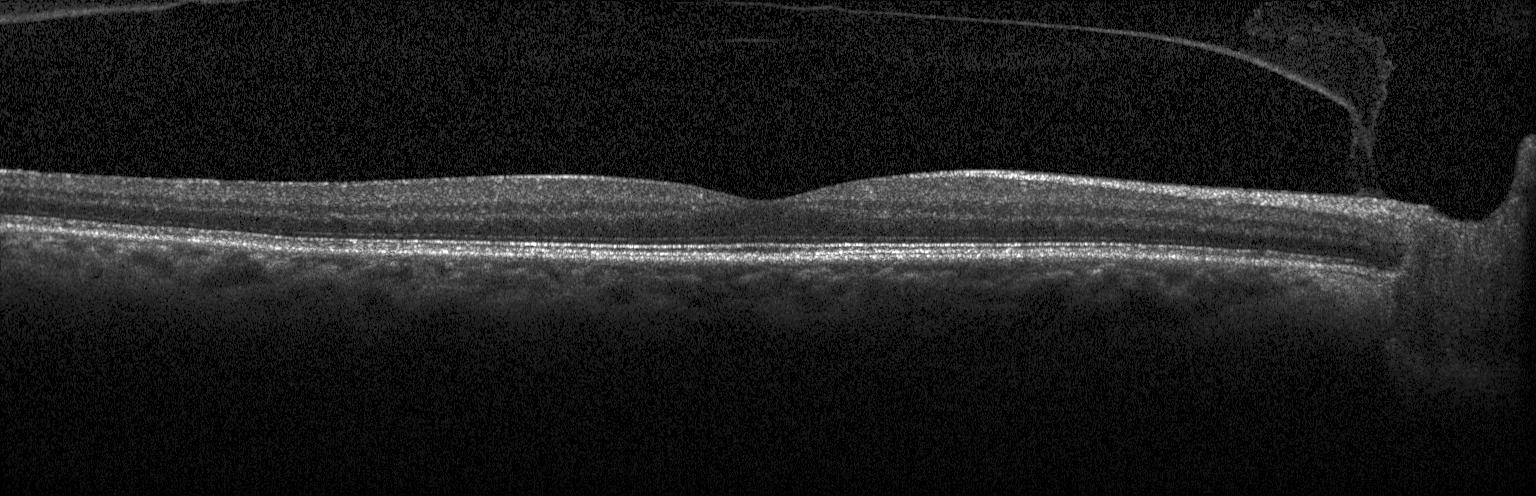

OCT line scan.
Assessment: no choroidal neovascularization, diabetic macular edema, or drusen.